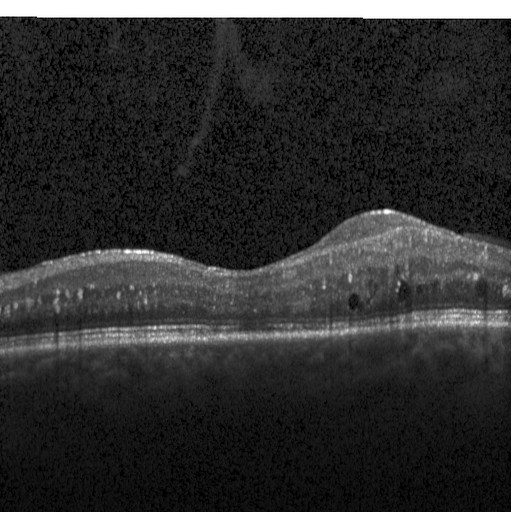

Retinal OCT B-scan. Acquired on a Heidelberg Spectralis. Finding: diabetic macular edema (DME).